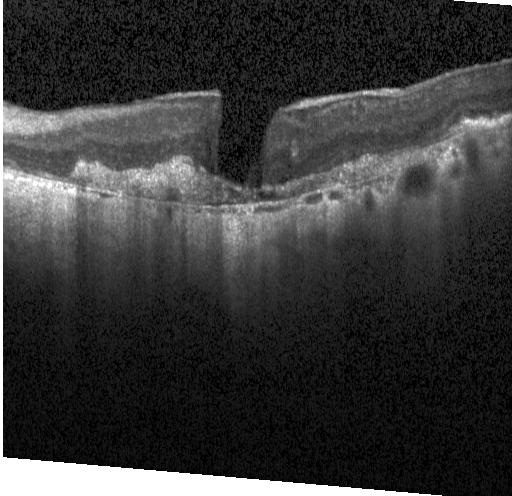 The scan shows CNV.